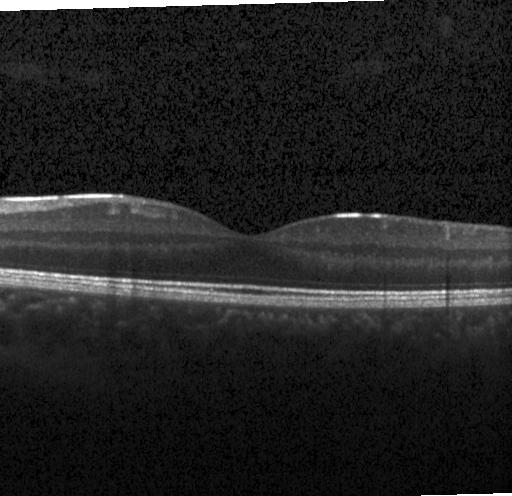 Macular OCT: no evidence of CNV, DME, or drusen.